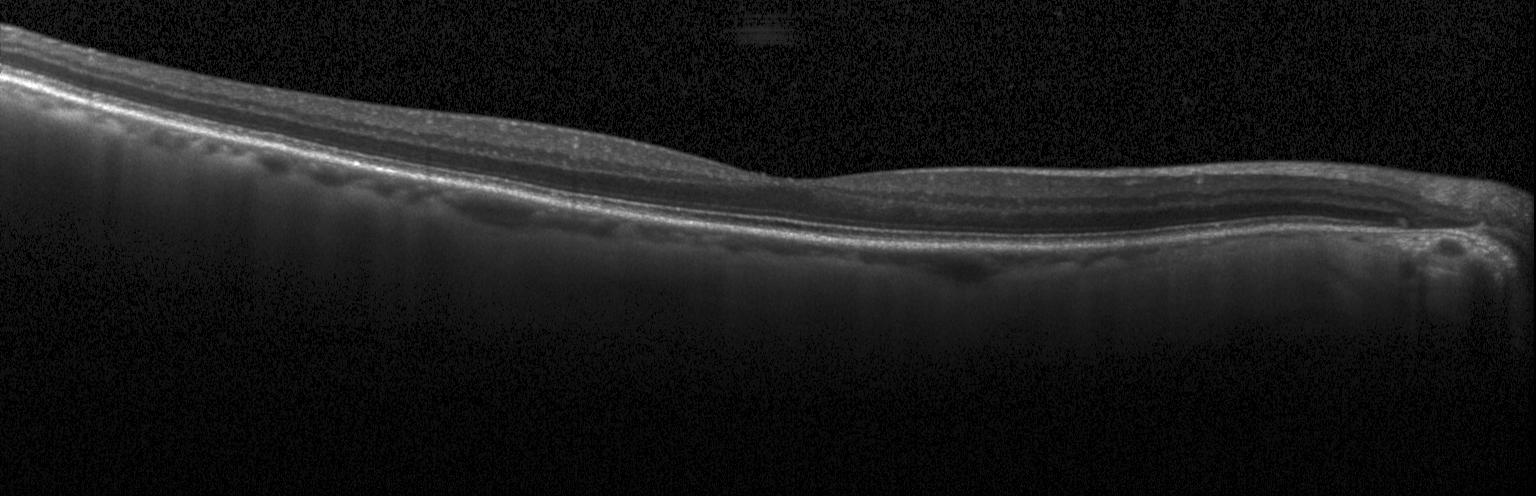
Centered on the fovea; retinal OCT B-scan — No evidence of choroidal neovascularization, diabetic macular edema, or drusen.